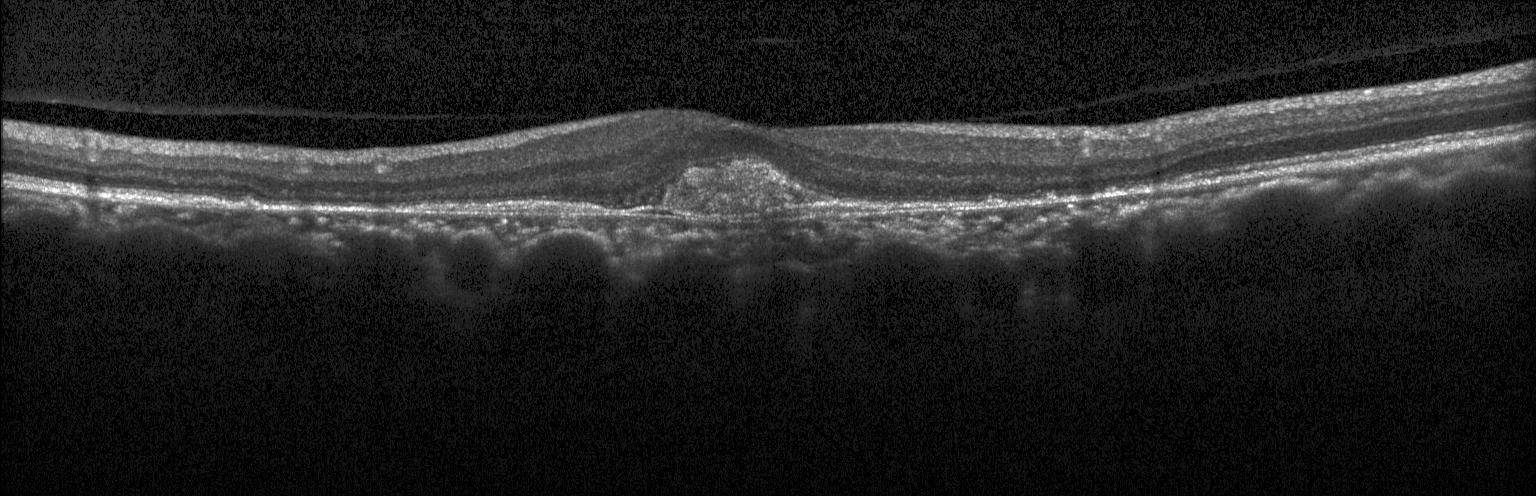

Optical coherence tomography B-scan. Spectral-domain OCT — Assessment: a choroidal neovascular membrane.